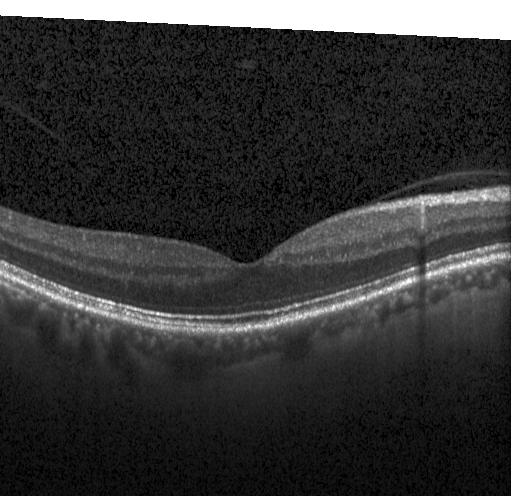

Retinal OCT cross-section — The scan shows no choroidal neovascularization, no diabetic macular edema, and no drusen.